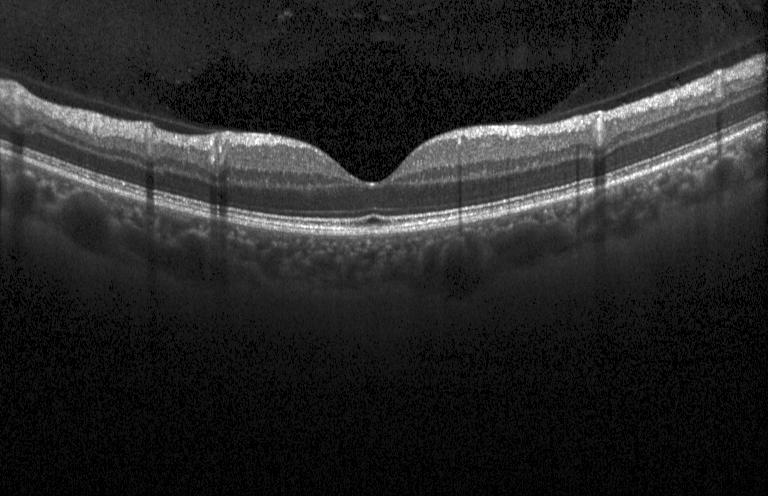 OCT B-scan
Assessment: neither CNV, DME, nor drusen.